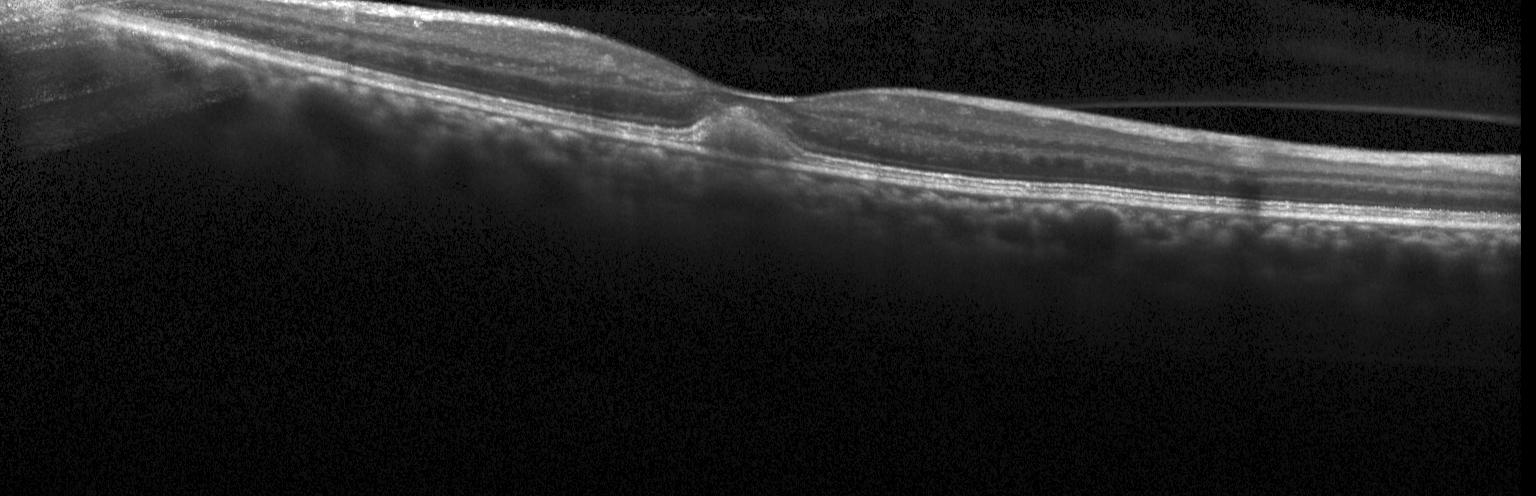
Finding: a choroidal neovascular membrane.